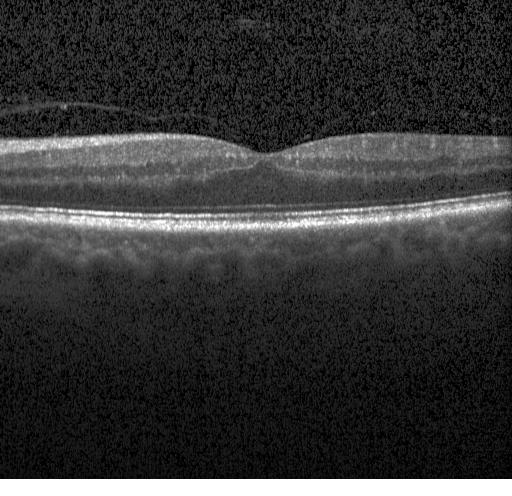 Retinal OCT B-scan. Heidelberg Spectralis OCT system.
Macular OCT: no choroidal neovascularization, no diabetic macular edema, and no drusen.